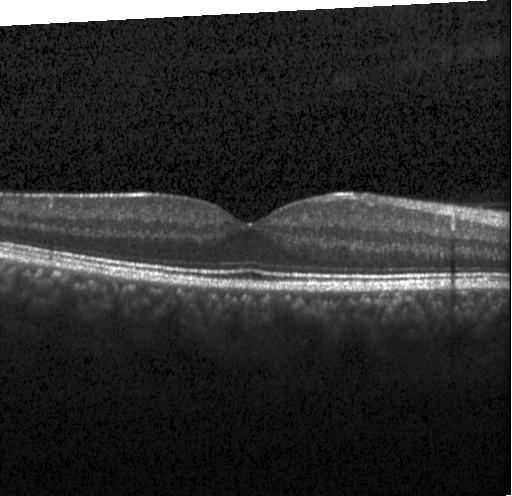
Retinal OCT B-scan.
Finding: no choroidal neovascularization, diabetic macular edema, or drusen.